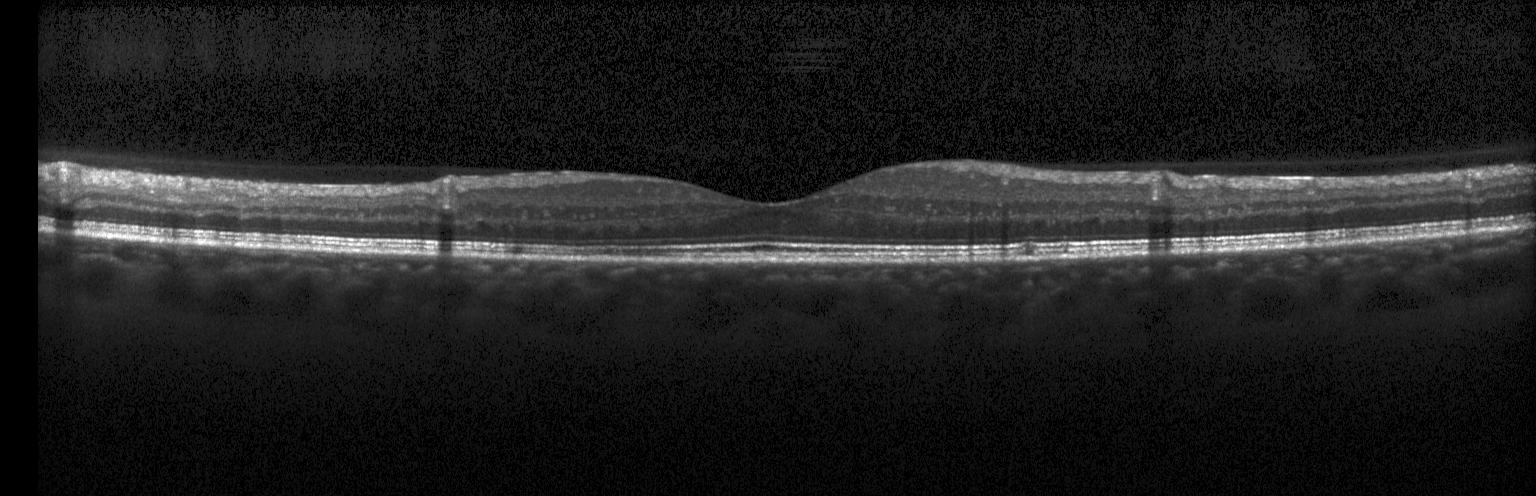

OCT B-scan
The scan shows no CNV, no DME, and no drusen.